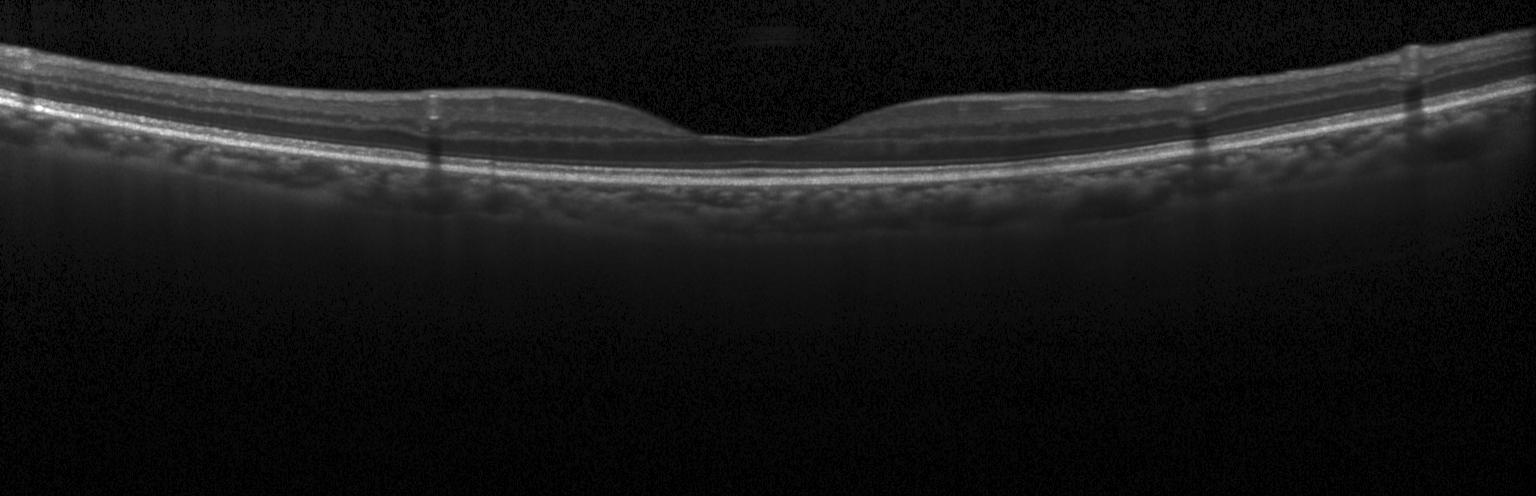 OCT line scan · spectral-domain optical coherence tomography. Macular OCT: no choroidal neovascularization, no diabetic macular edema, and no drusen.